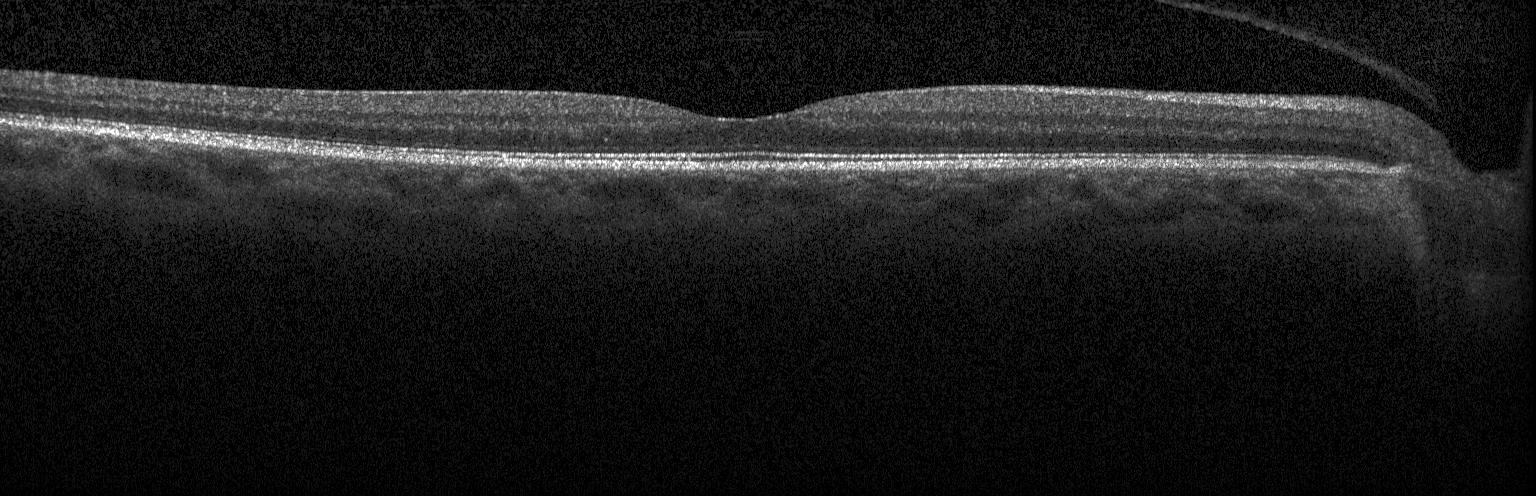 Retinal OCT cross-section, instrument: Heidelberg Spectralis. The scan shows no choroidal neovascularization, no diabetic macular edema, and no drusen.